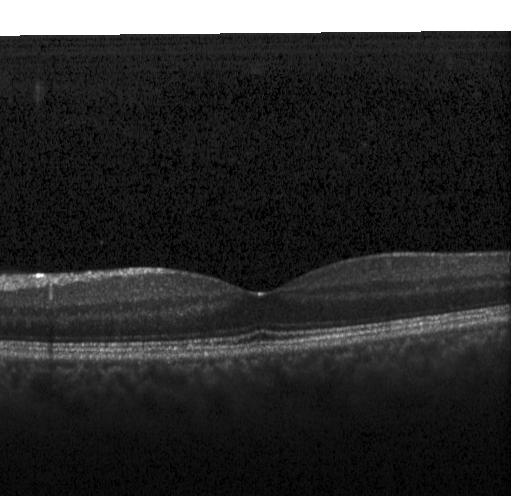 Centered on the fovea; optical coherence tomography B-scan
Assessment: no choroidal neovascularization, no diabetic macular edema, and no drusen.